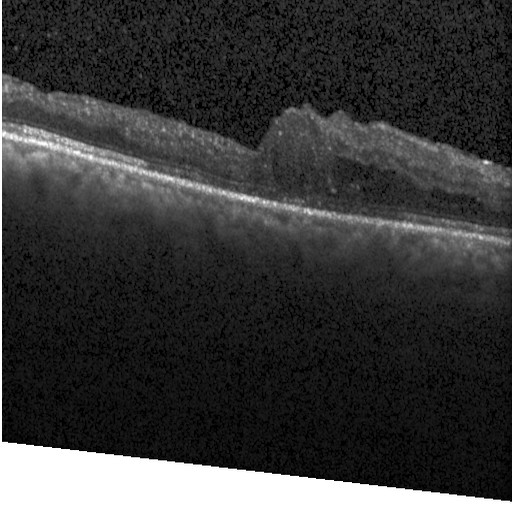 Retinal OCT cross-section. Impression: diabetic macular edema (DME).